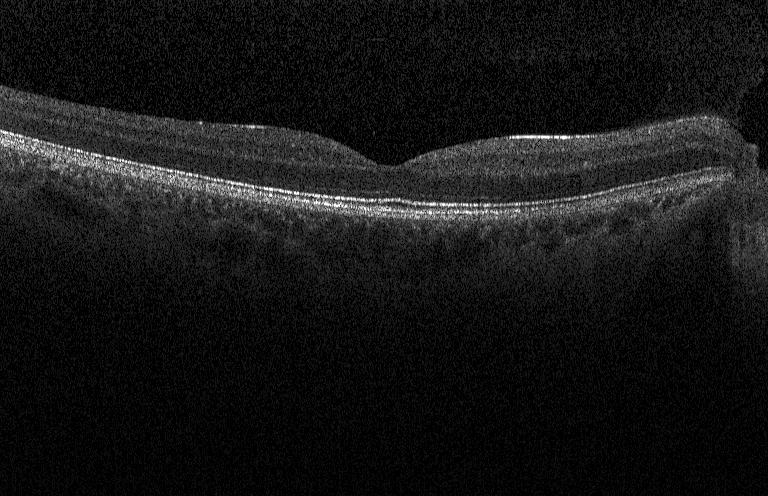
The scan shows no choroidal neovascularization, no diabetic macular edema, and no drusen.